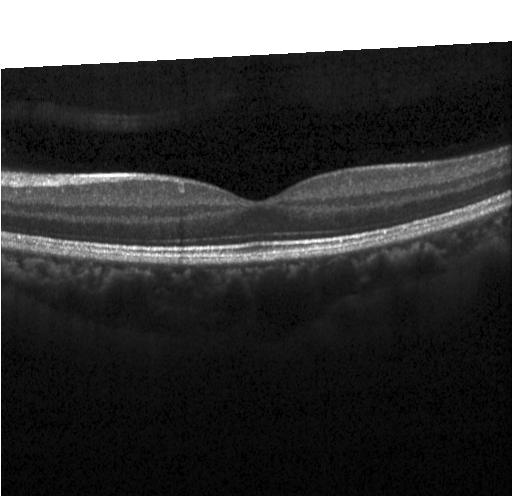 OCT line scan
OCT finding: no choroidal neovascularization, no diabetic macular edema, and no drusen.